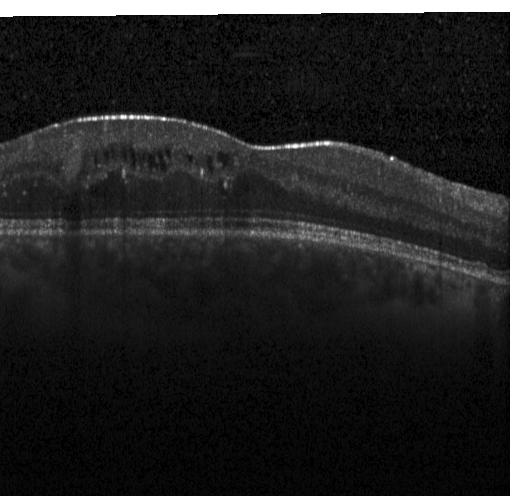

OCT B-scan.
This B-scan demonstrates DME.